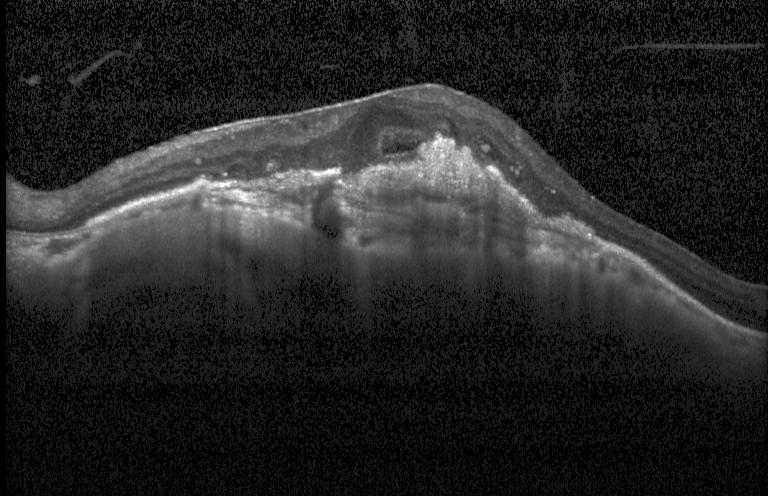 Finding: choroidal neovascularization (CNV).